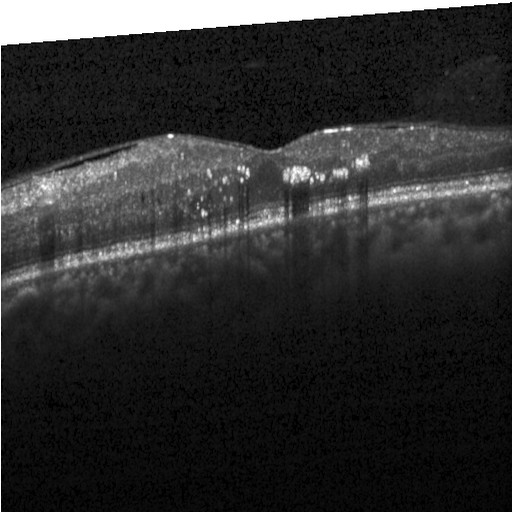 OCT scan showing DME.